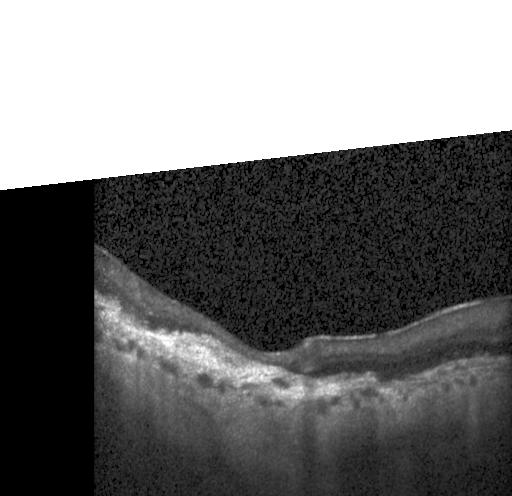
Optical coherence tomography scan; SD-OCT — Choroidal neovascularization (CNV).